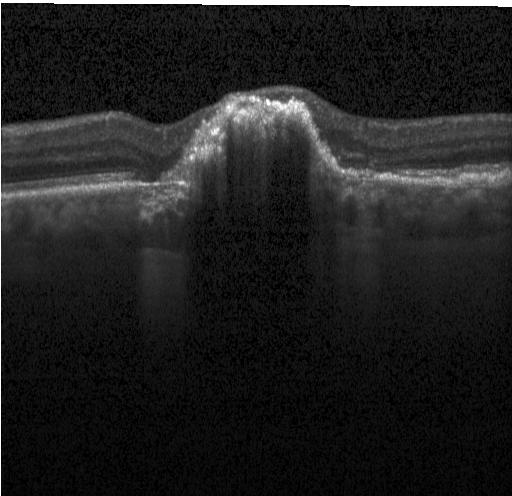
Finding: CNV.